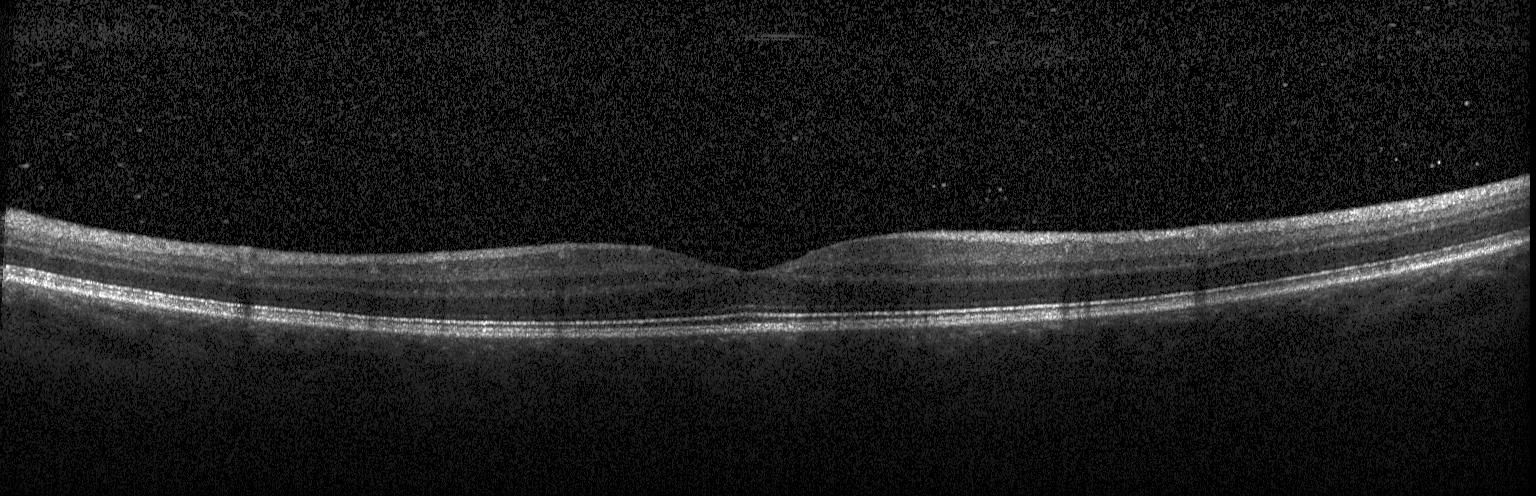
Retinal OCT cross-section showing neither choroidal neovascularization, diabetic macular edema, nor drusen.